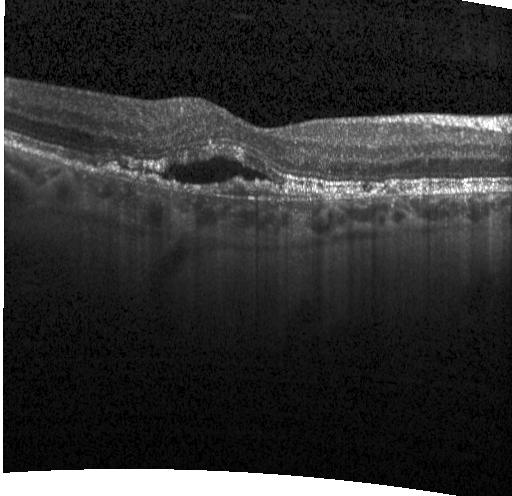
Finding: a choroidal neovascular membrane.